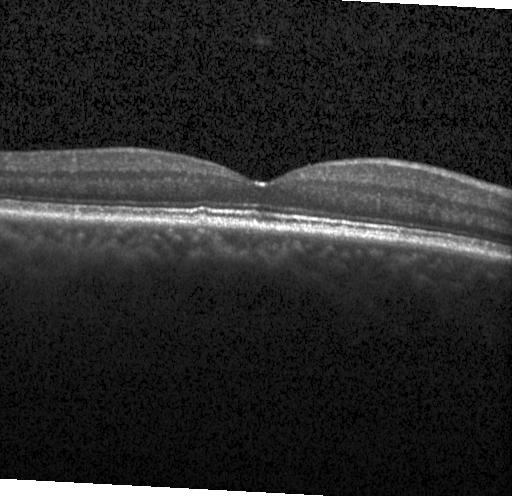 Instrument: Heidelberg Spectralis. Retinal OCT cross-section — Neither choroidal neovascularization, diabetic macular edema, nor drusen.